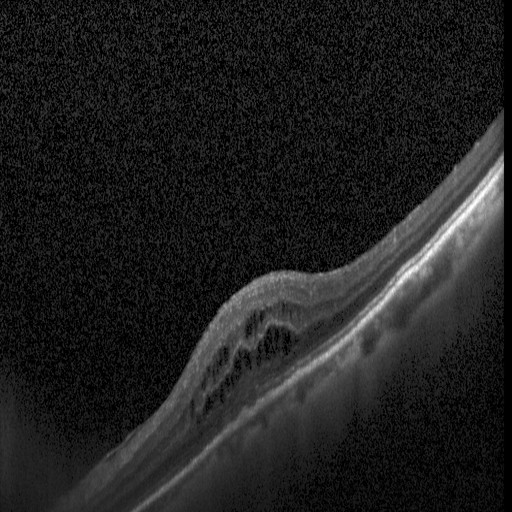
Optical coherence tomography B-scan; macular scan; SD-OCT; acquired on a Heidelberg Spectralis. Diagnosis: diabetic macular edema.